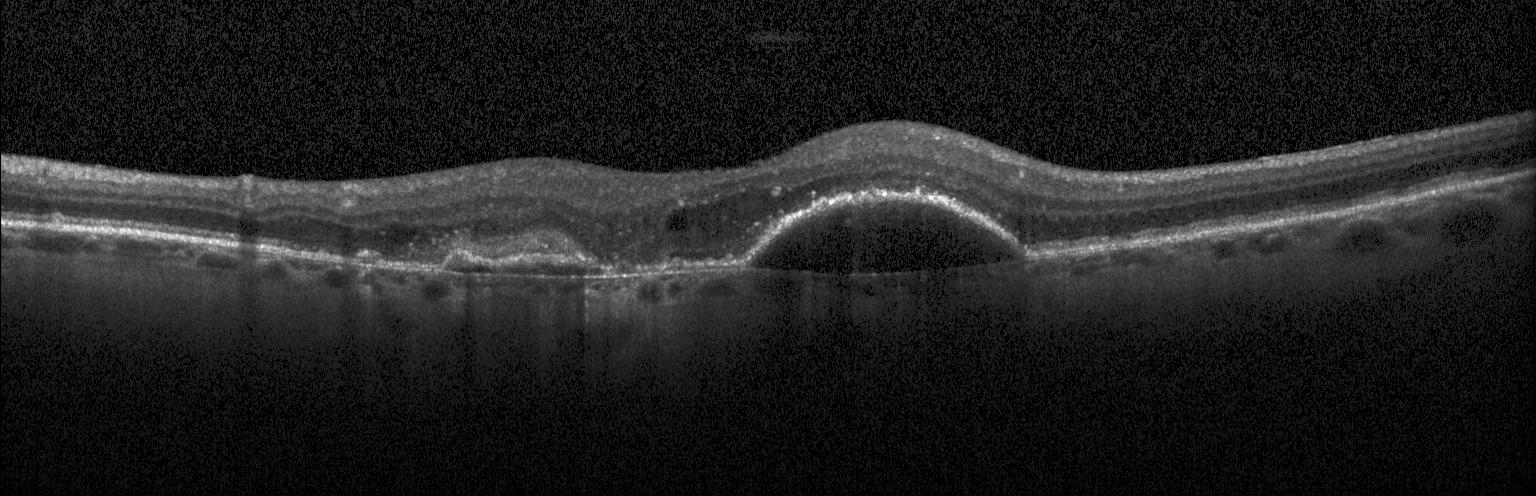
OCT finding: choroidal neovascularization.